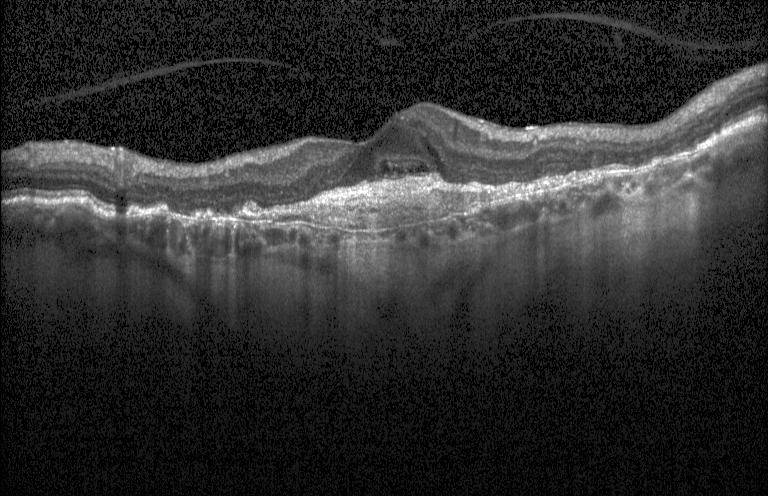

Spectral-domain optical coherence tomography. Optical coherence tomography scan. Heidelberg Spectralis OCT system.
Impression: choroidal neovascularization (CNV).